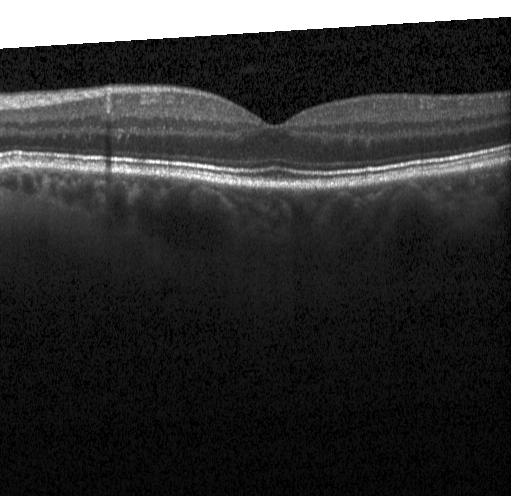
Retinal OCT B-scan.
No evidence of CNV, DME, or drusen.